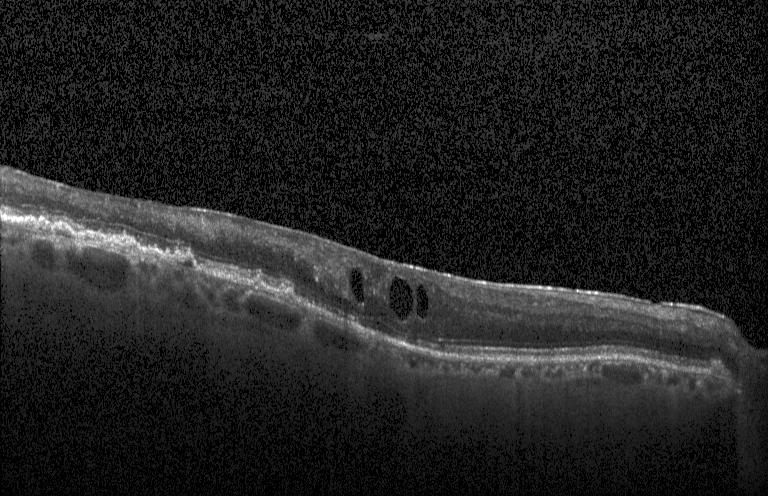

Macular OCT: choroidal neovascularization (CNV).